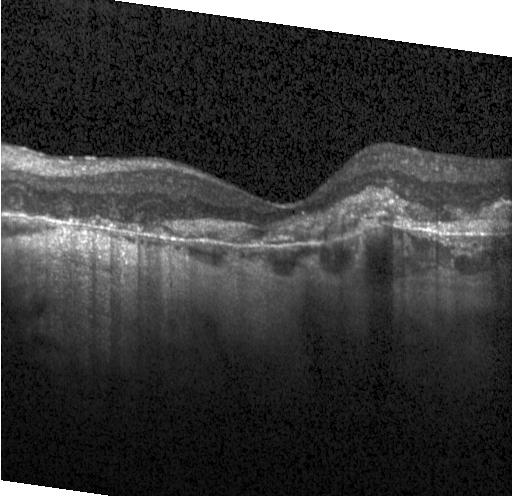

Instrument: Heidelberg Spectralis · optical coherence tomography scan
OCT finding: CNV.